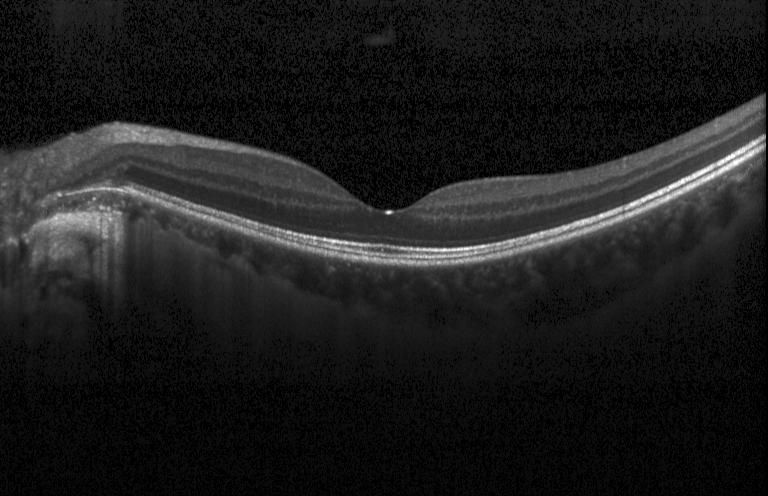
Retinal OCT B-scan · macular scan.
Assessment: no evidence of choroidal neovascularization, diabetic macular edema, or drusen.